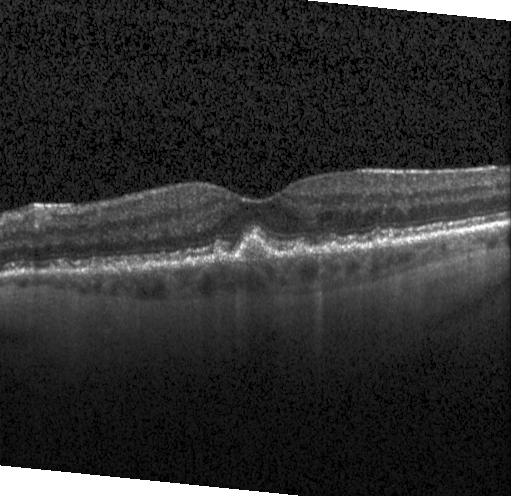 Through the macula · OCT line scan · SD-OCT. Assessment: drusen.